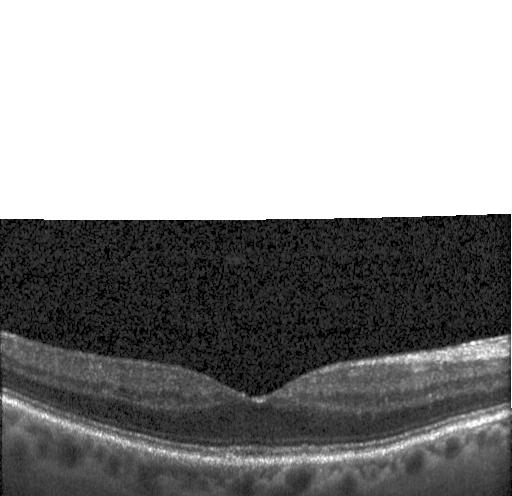
Diagnosis: no CNV, DME, or drusen.